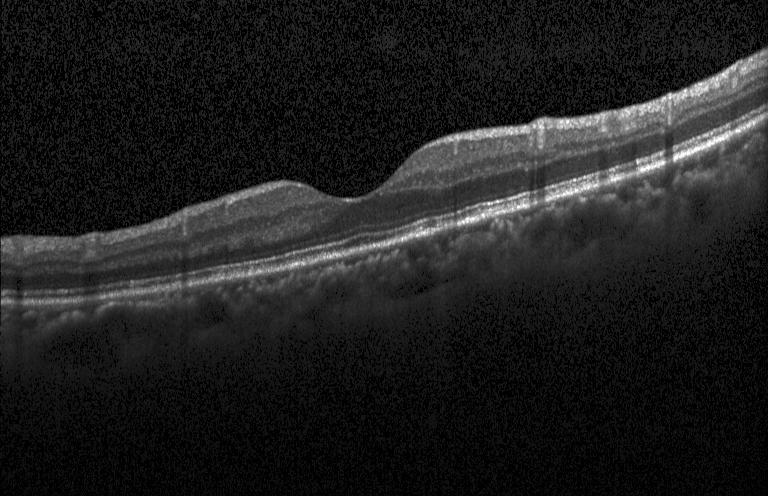

Retinal OCT cross-section showing no choroidal neovascularization, no diabetic macular edema, and no drusen.